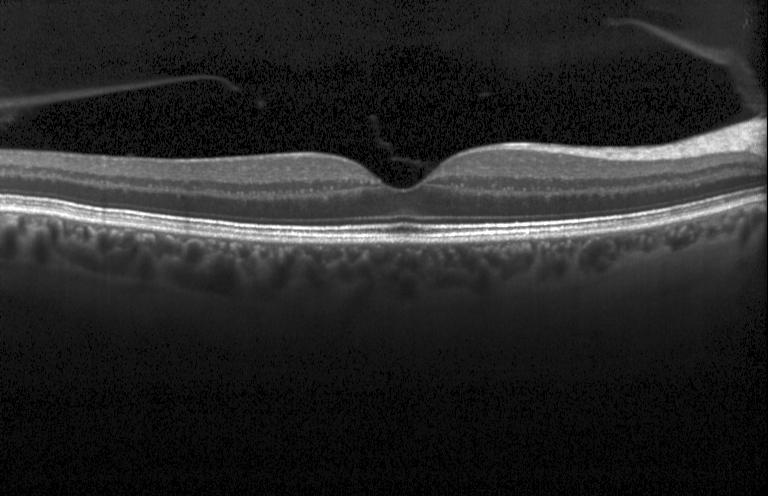 Acquired on a Heidelberg Spectralis; SD-OCT; optical coherence tomography scan.
The scan shows neither choroidal neovascularization, diabetic macular edema, nor drusen.